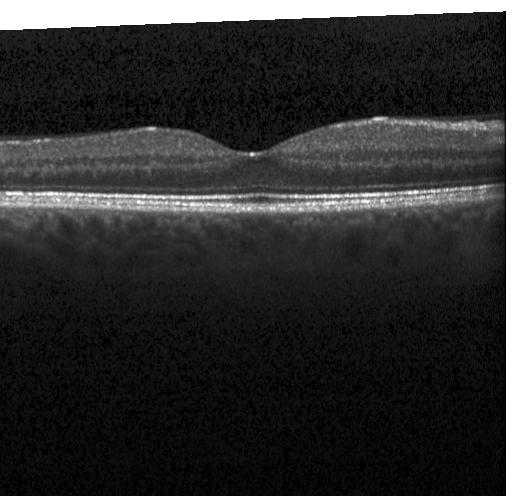

OCT finding: no evidence of CNV, DME, or drusen.